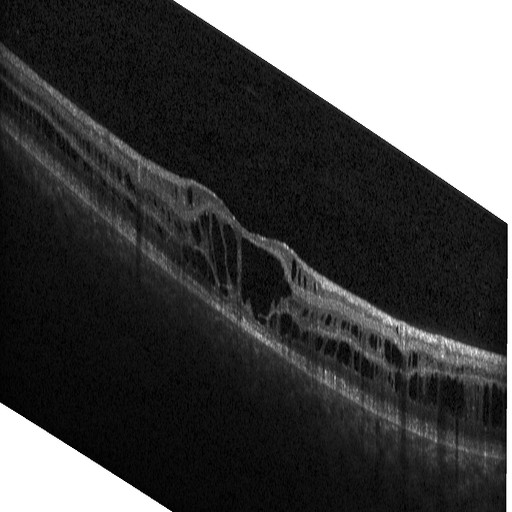
OCT line scan — OCT finding: diabetic macular edema.